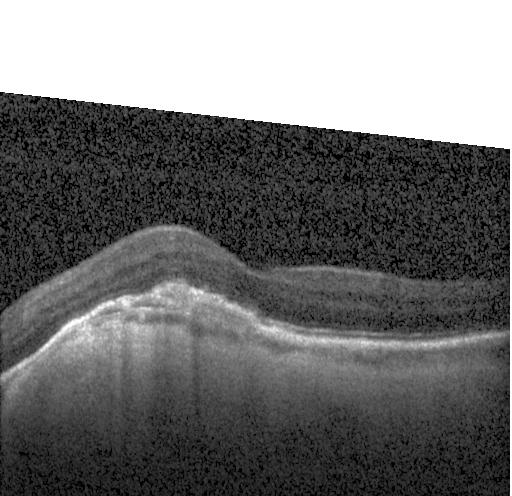
OCT B-scan; fovea-centered; spectral-domain OCT — Dx: choroidal neovascularization (CNV).